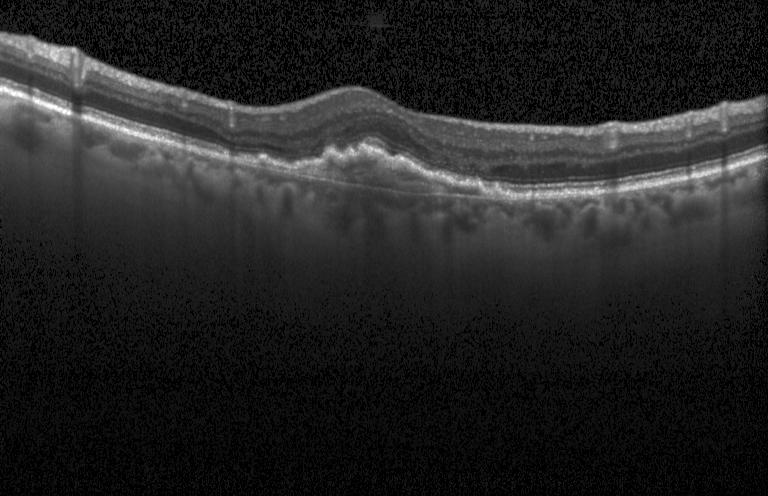 Optical coherence tomography B-scan. Instrument: Heidelberg Spectralis. Centered on the fovea. Spectral-domain OCT
Finding: a choroidal neovascular membrane.